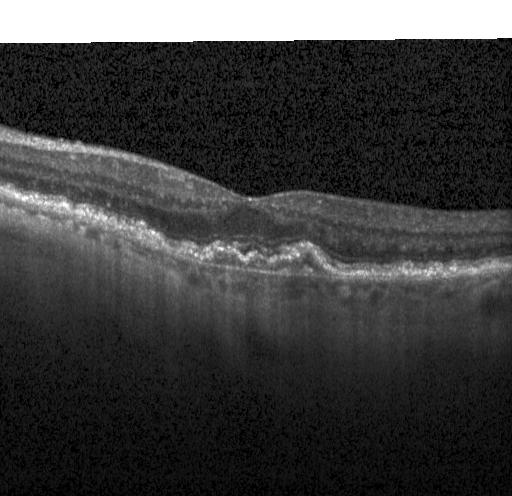
Optical coherence tomography scan. Fovea-centered. Acquired on a Heidelberg Spectralis.
Dx: a choroidal neovascular membrane.